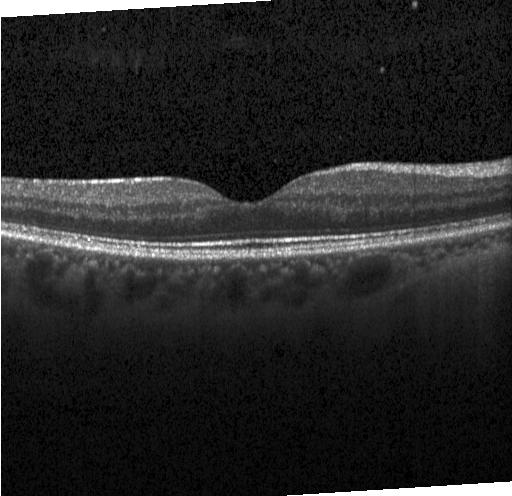
Impression: no CNV, no DME, and no drusen.